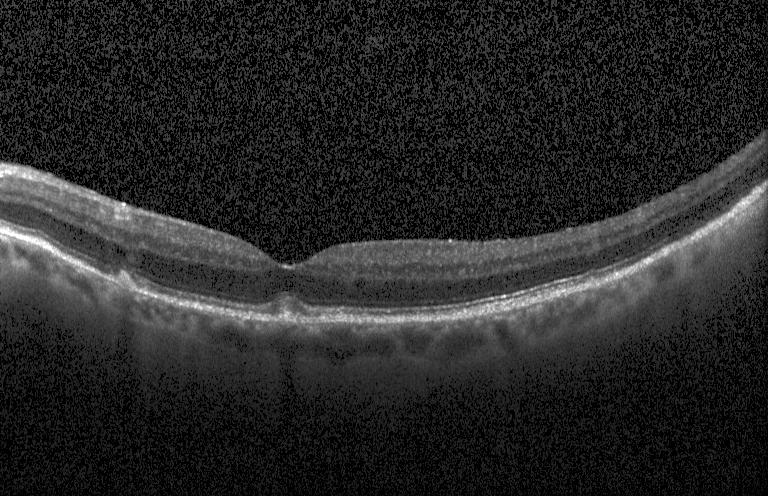

Retinal OCT cross-section — Impression: multiple drusen.